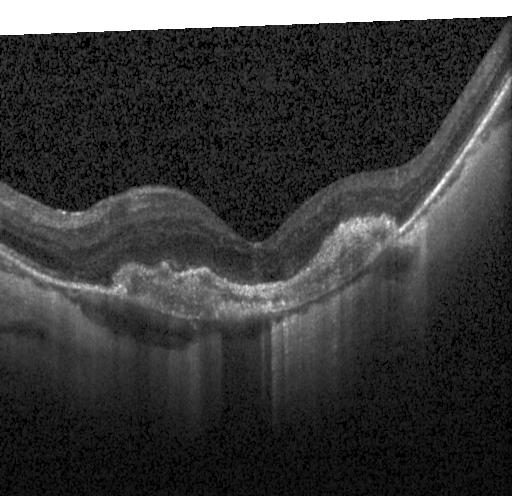 Instrument: Heidelberg Spectralis. Spectral-domain optical coherence tomography. Retinal OCT B-scan. Fovea-centered.
OCT finding: choroidal neovascularization.